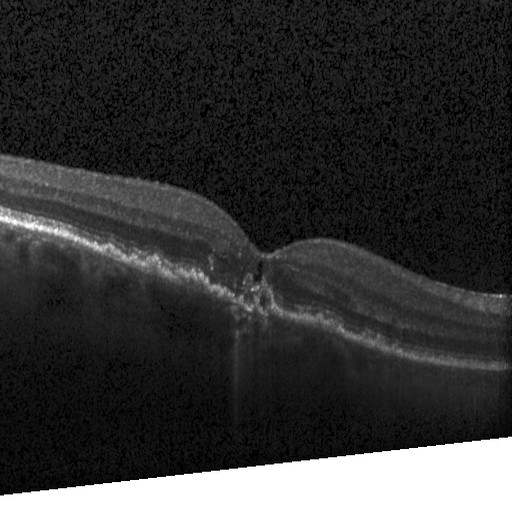

OCT B-scan · instrument: Heidelberg Spectralis. The scan shows DME.